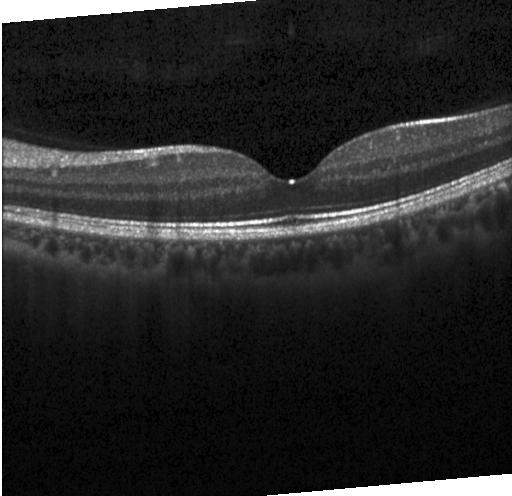 Retinal OCT cross-section showing no evidence of choroidal neovascularization, diabetic macular edema, or drusen.